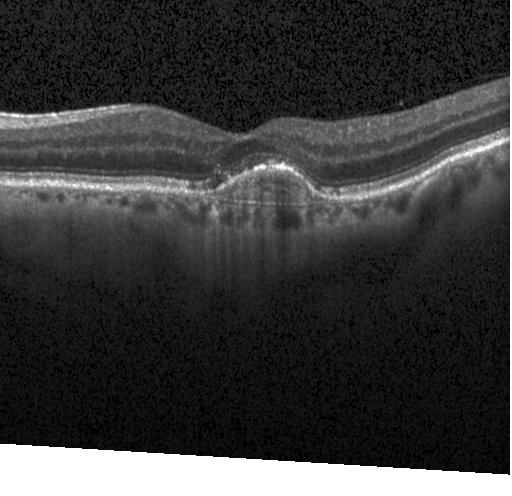 Optical coherence tomography B-scan.
Diagnosis: a choroidal neovascular membrane.